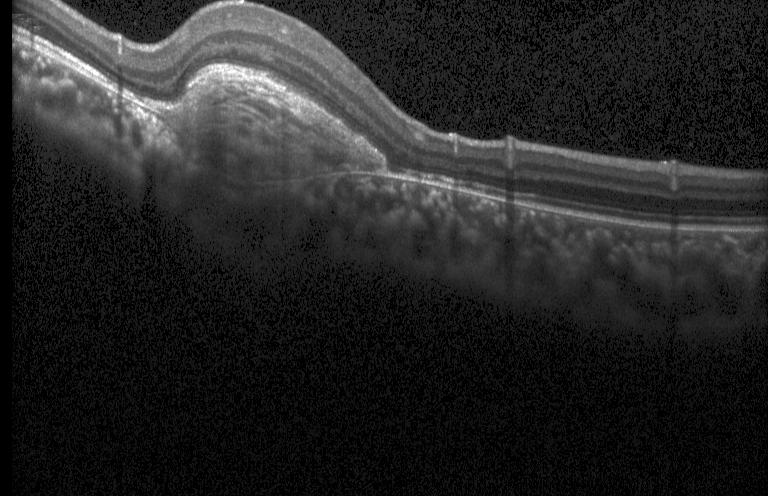

OCT finding: choroidal neovascularization (CNV).